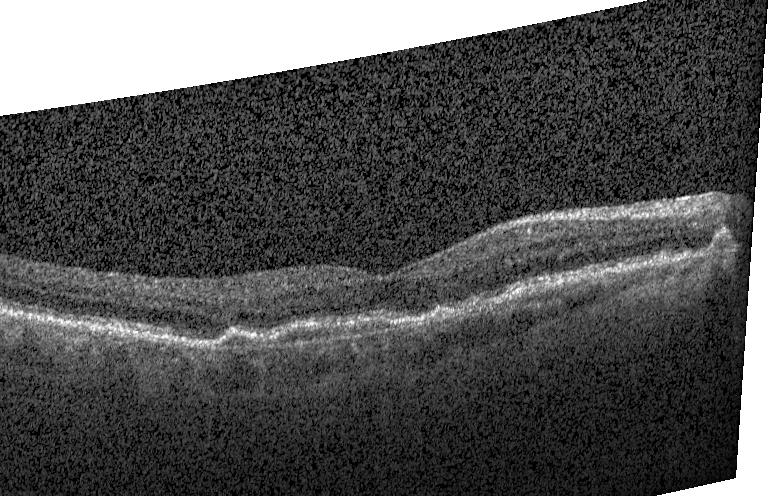 Retinal OCT cross-section · SD-OCT · Heidelberg Spectralis · horizontal scan through the fovea
The scan shows choroidal neovascularization (CNV).